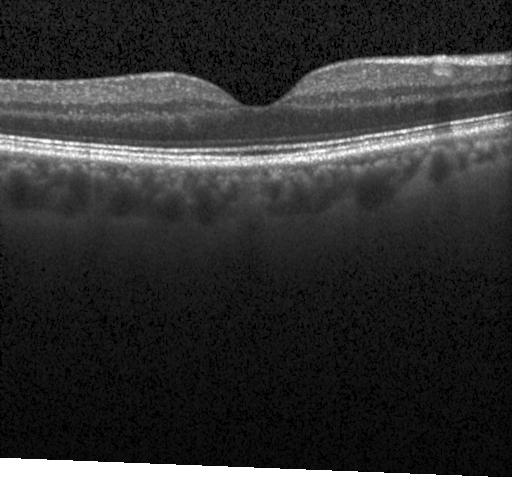
Optical coherence tomography B-scan. Finding: no choroidal neovascularization, diabetic macular edema, or drusen.